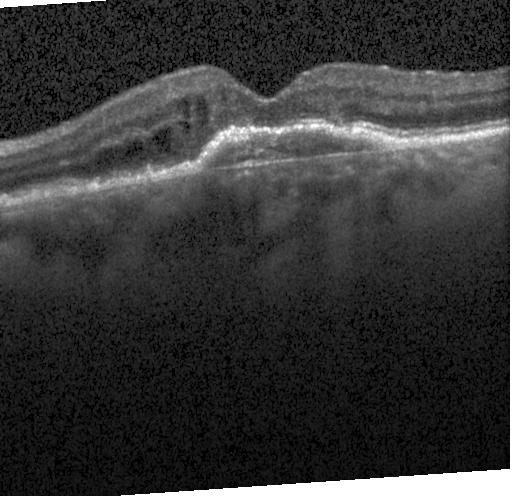

Through the macula · spectral-domain optical coherence tomography · retinal OCT cross-section · Heidelberg Spectralis — Macular OCT: CNV.